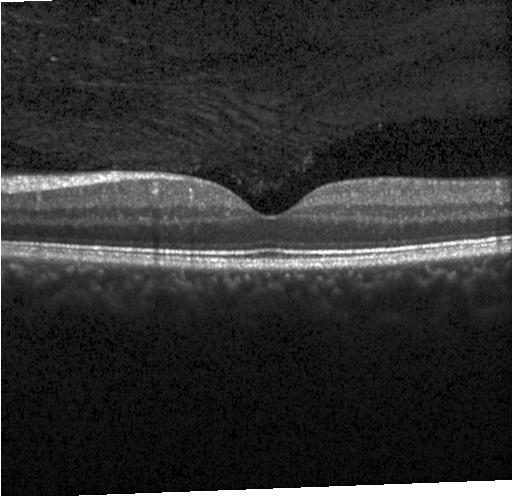
OCT scan showing no choroidal neovascularization, no diabetic macular edema, and no drusen.